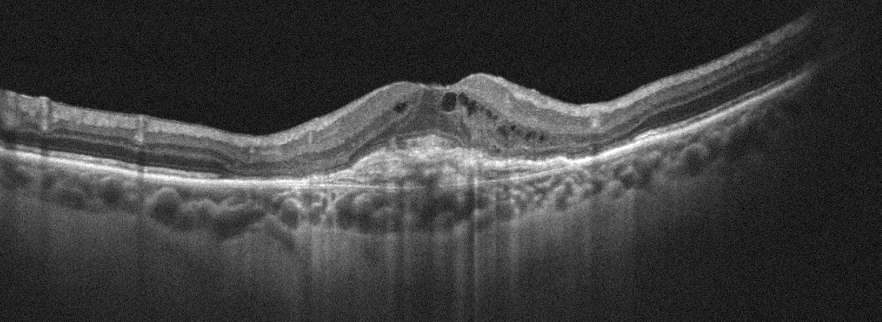

Right eye, acquired on an Optovue Avanti RTVue XR, macular scan, retinal OCT B-scan. Assessment: age-related macular degeneration (AMD).